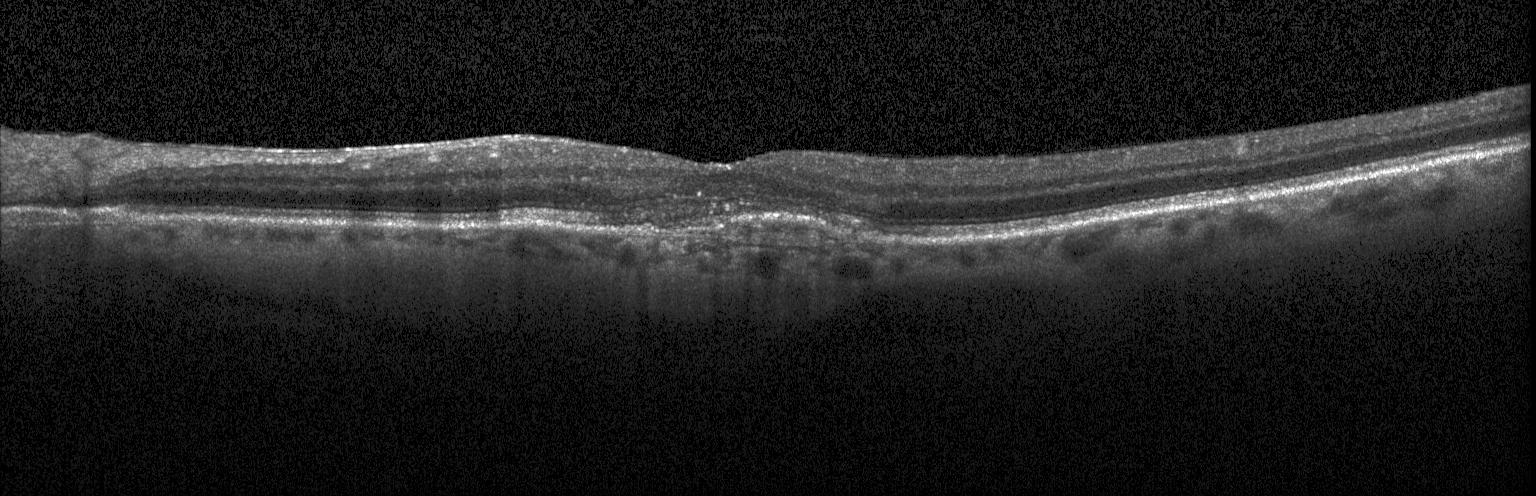

Spectral-domain OCT; retinal OCT cross-section; horizontal scan through the fovea; Heidelberg Spectralis.
Finding: choroidal neovascularization.